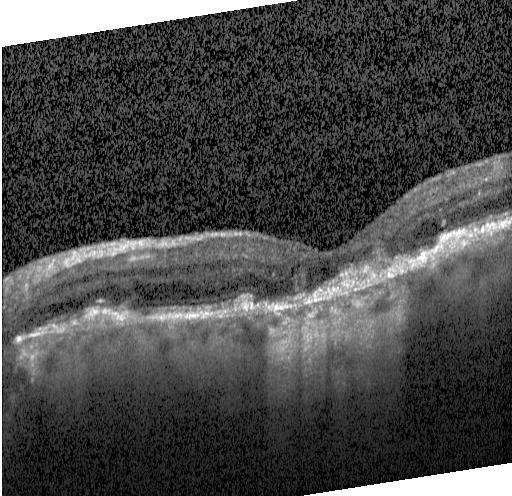 Optical coherence tomography scan. Macular scan. SD-OCT. Acquired on a Heidelberg Spectralis. Assessment: choroidal neovascularization (CNV).